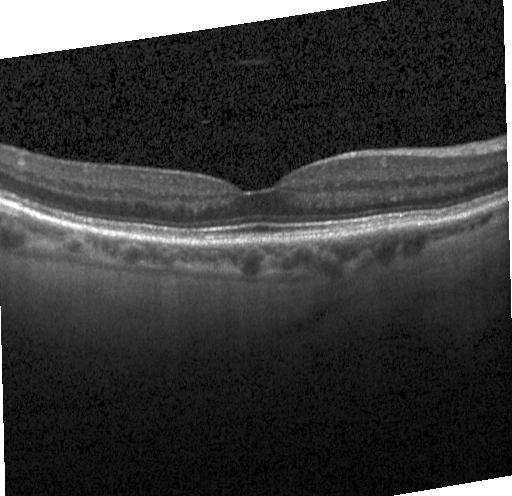 Optical coherence tomography B-scan. Through the macula — The scan shows no CNV, DME, or drusen.